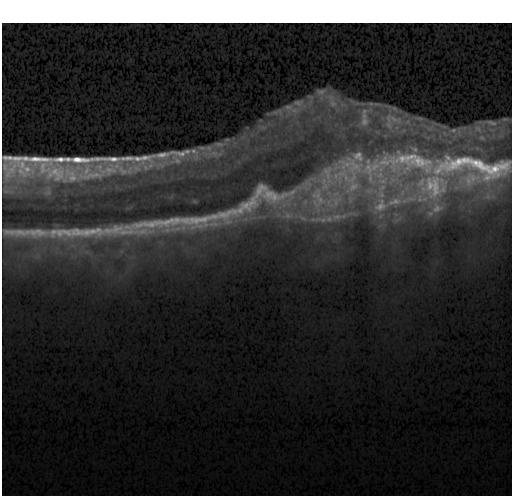

OCT line scan
Finding: choroidal neovascularization.